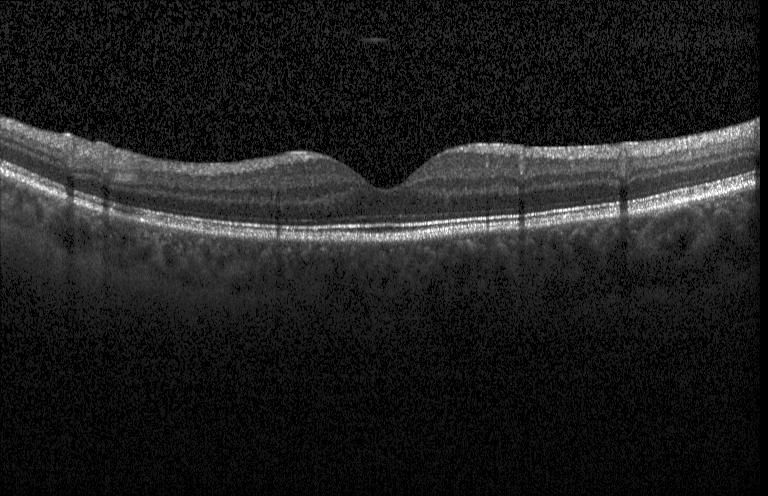
Through the macula. Optical coherence tomography scan. Instrument: Heidelberg Spectralis.
Impression: neither choroidal neovascularization, diabetic macular edema, nor drusen.